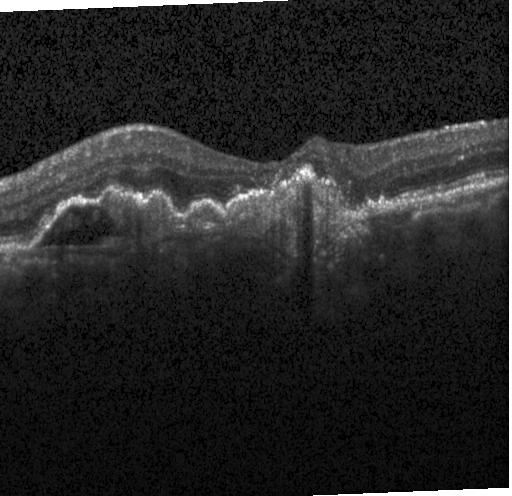
Retinal OCT cross-section showing choroidal neovascularization.